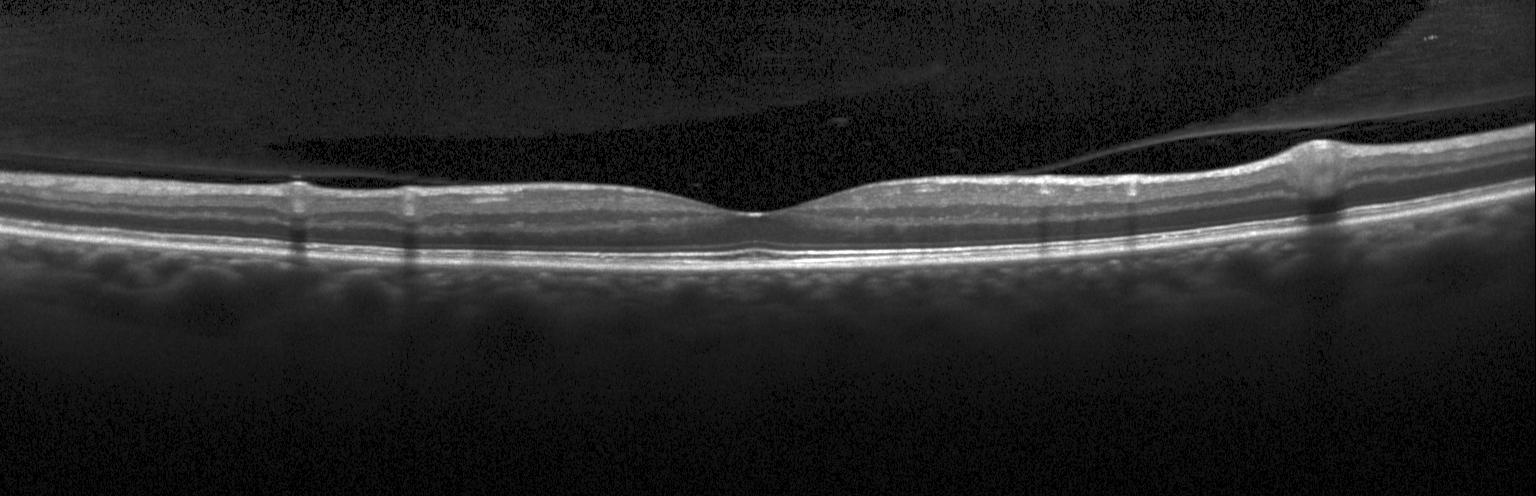
Horizontal scan through the fovea; retinal OCT cross-section. Assessment: no CNV, no DME, and no drusen.